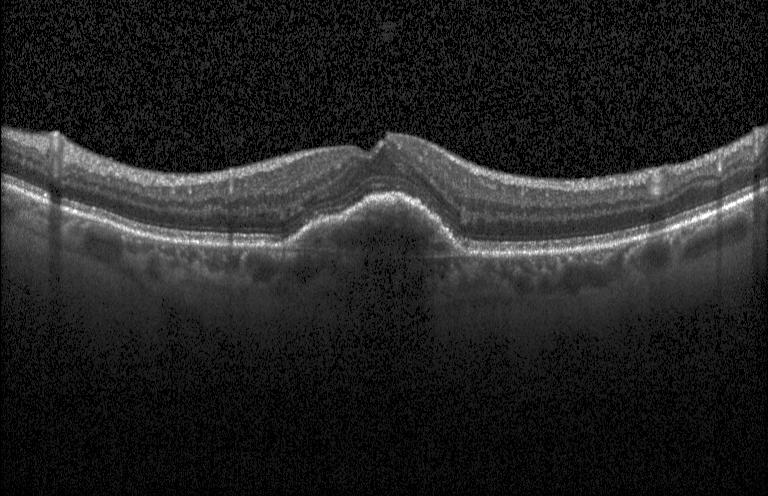
Macular OCT: choroidal neovascularization.